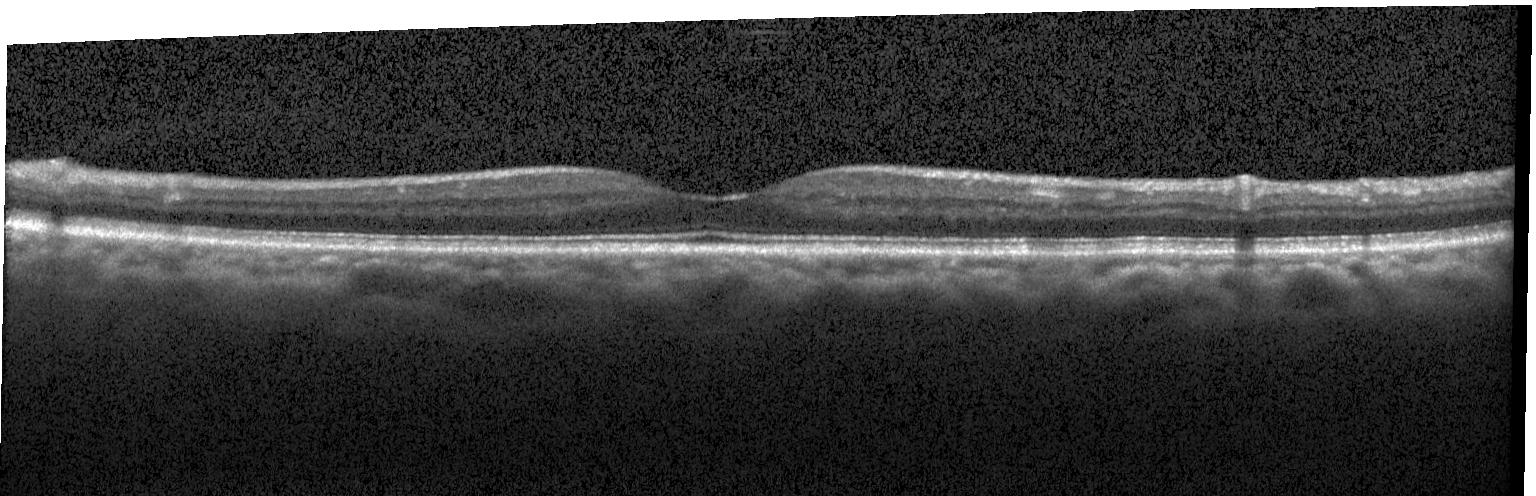
Macular scan, optical coherence tomography scan, acquired on a Heidelberg Spectralis.
OCT finding: no choroidal neovascularization, no diabetic macular edema, and no drusen.